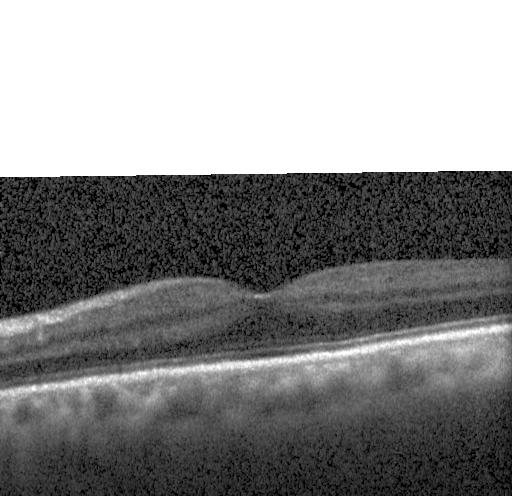
Diagnosis: neither CNV, DME, nor drusen.